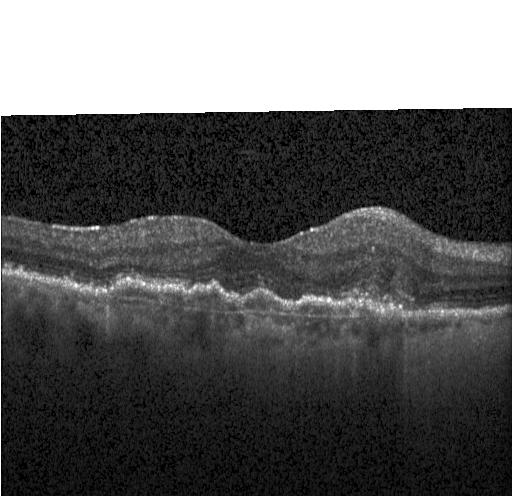

Assessment: CNV.